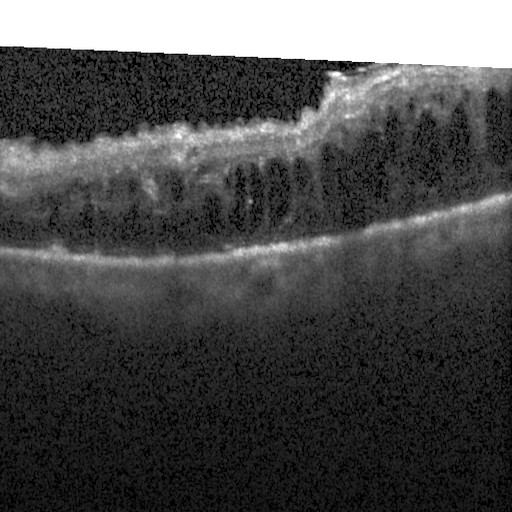 Diabetic macular edema (DME).